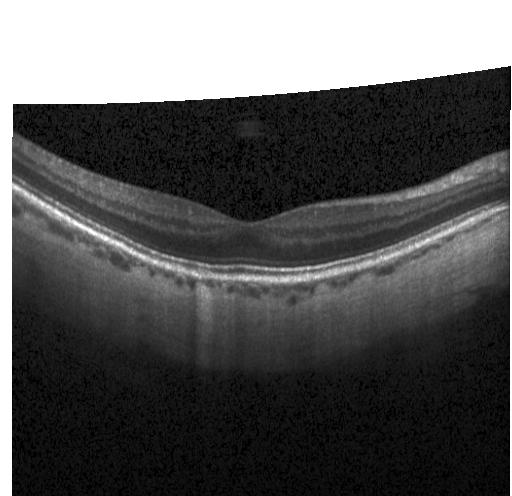

SD-OCT · optical coherence tomography B-scan
OCT finding: no CNV, DME, or drusen.